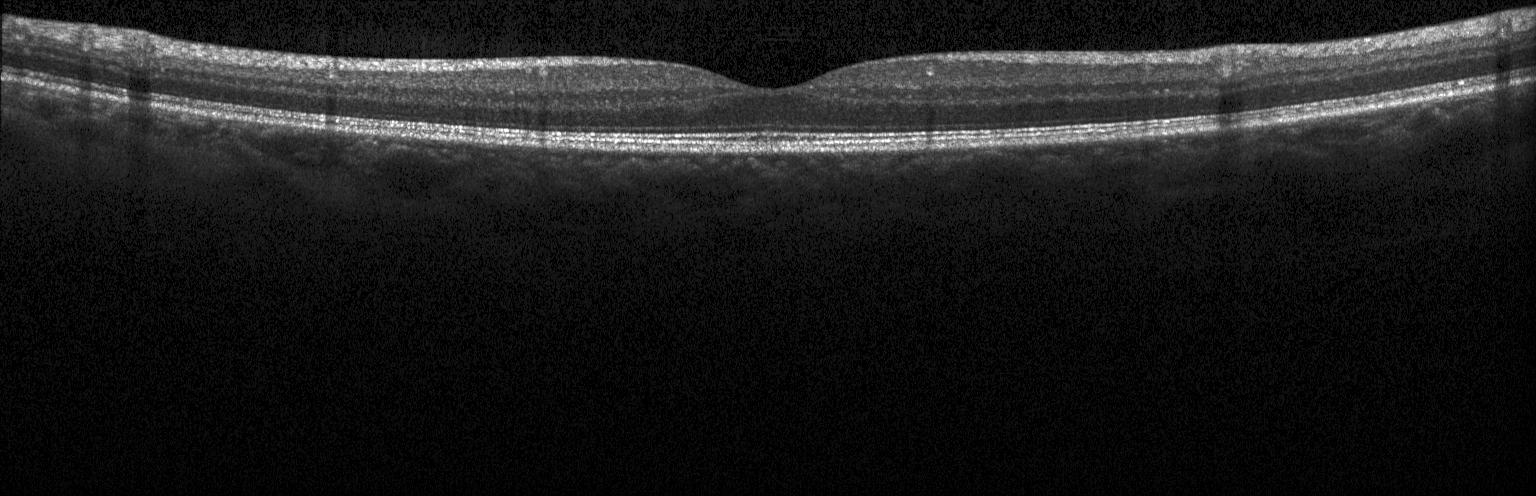

Impression: no CNV, DME, or drusen.